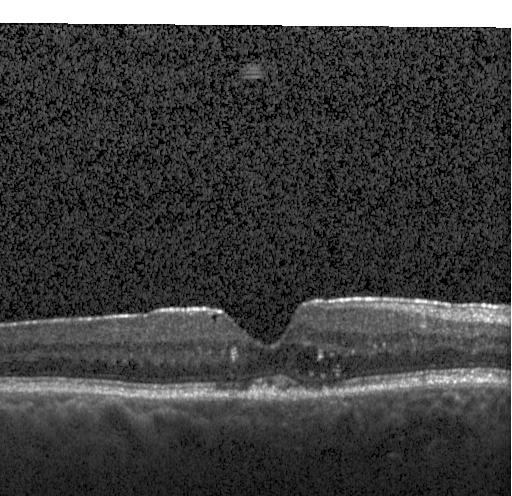
Macular OCT demonstrating a choroidal neovascular membrane.